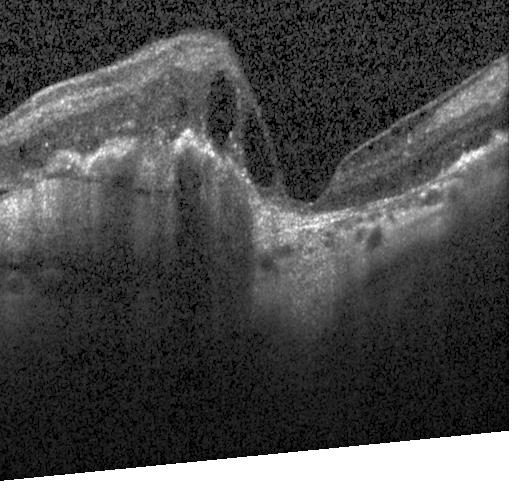 Instrument: Heidelberg Spectralis; horizontal scan through the fovea; optical coherence tomography B-scan — This B-scan demonstrates choroidal neovascularization (CNV).